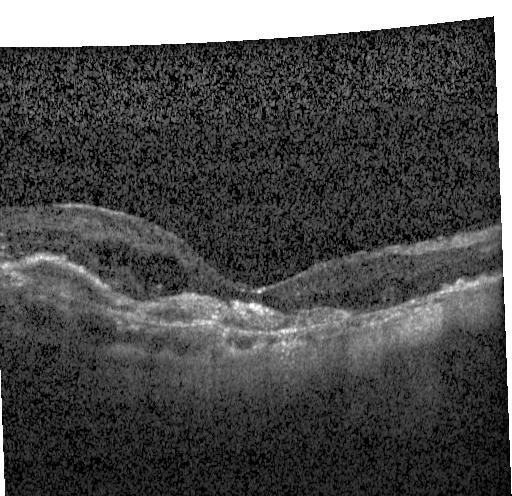
Retinal OCT B-scan; spectral-domain OCT; Heidelberg Spectralis OCT system. Impression: choroidal neovascularization (CNV).